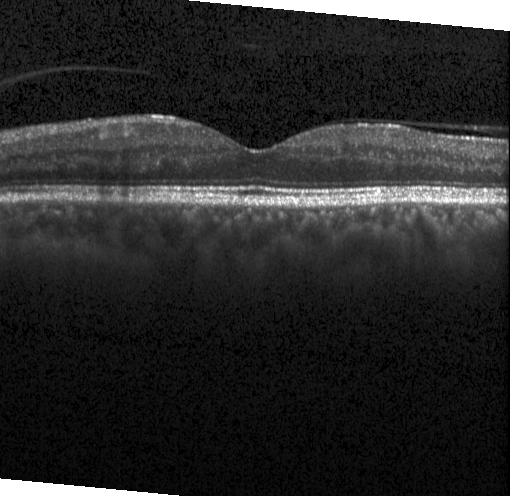

OCT scan showing no choroidal neovascularization, no diabetic macular edema, and no drusen.